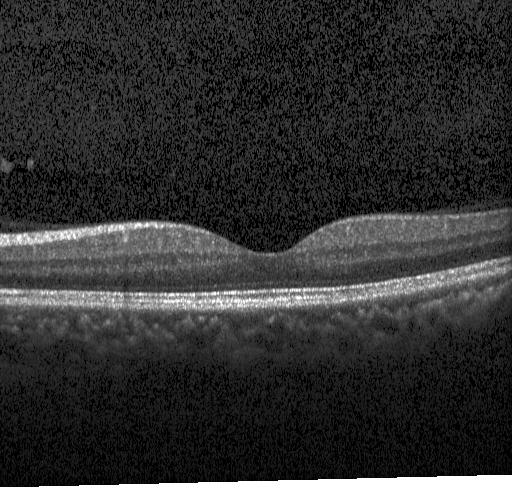
Neither choroidal neovascularization, diabetic macular edema, nor drusen.